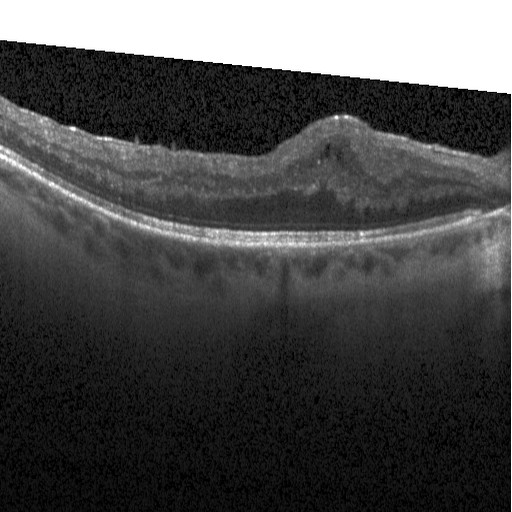
This B-scan demonstrates diabetic macular edema.